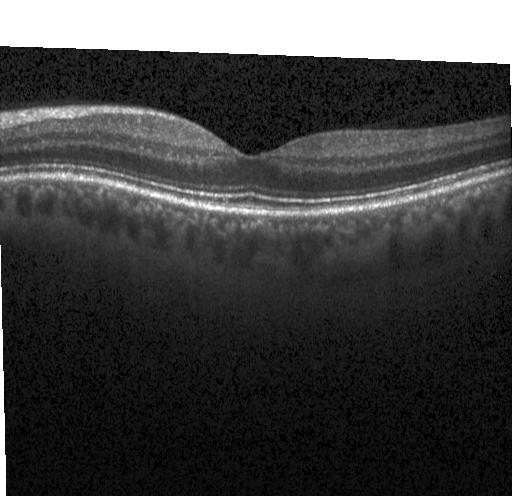

Spectral-domain OCT B-scan: no choroidal neovascularization, diabetic macular edema, or drusen.